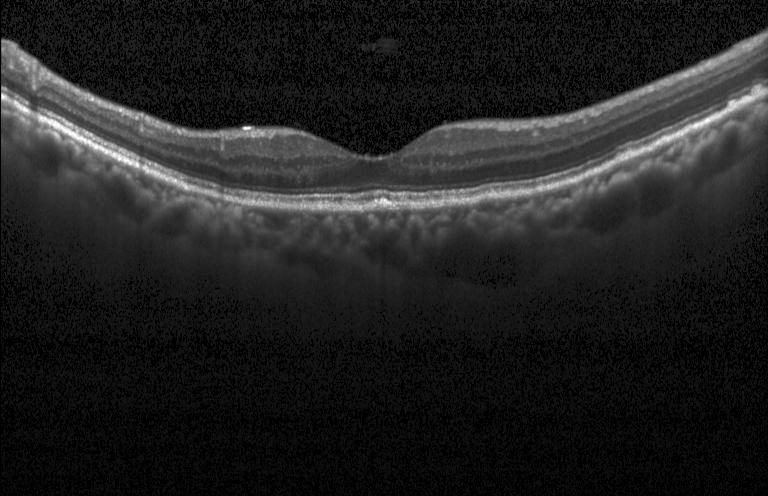 Retinal OCT cross-section — Finding: no choroidal neovascularization, diabetic macular edema, or drusen.